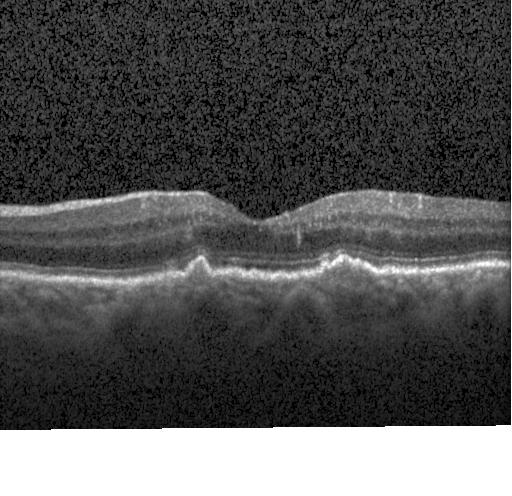

OCT B-scan. Diagnosis: drusen.